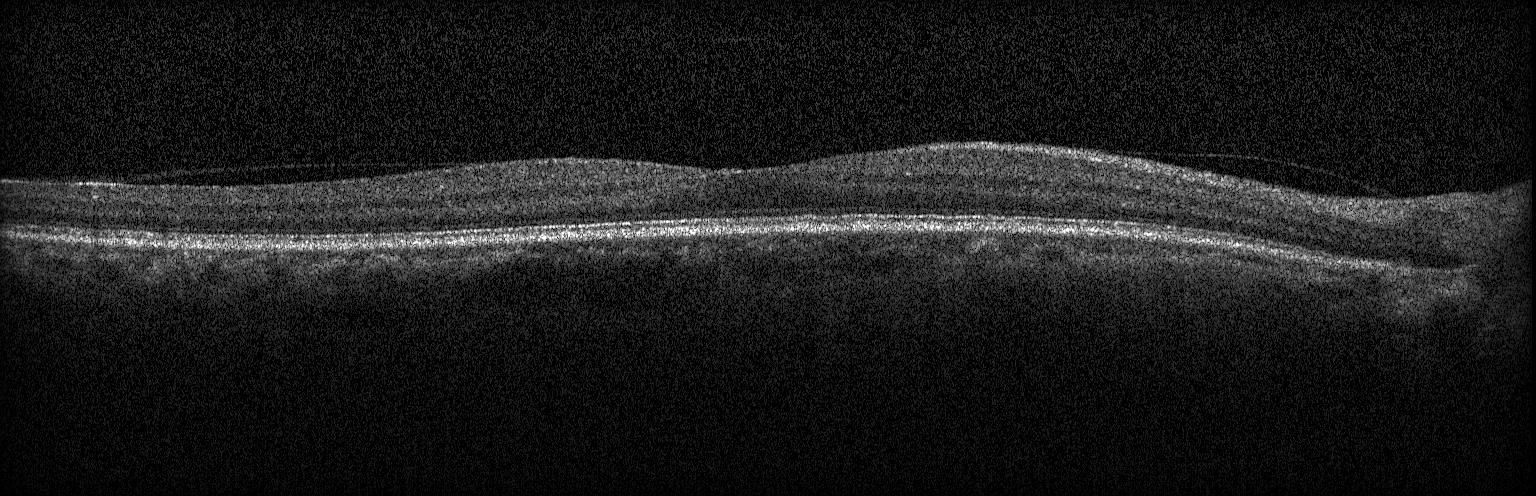

Retinal OCT cross-section; SD-OCT. Finding: neither choroidal neovascularization, diabetic macular edema, nor drusen.